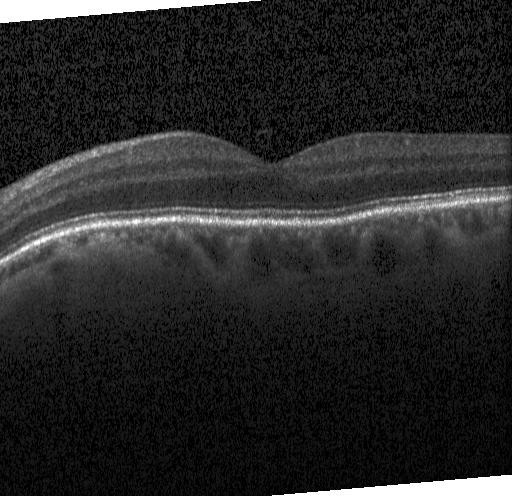 Retinal OCT cross-section; spectral-domain OCT; through the macula; instrument: Heidelberg Spectralis
Impression: no evidence of choroidal neovascularization, diabetic macular edema, or drusen.